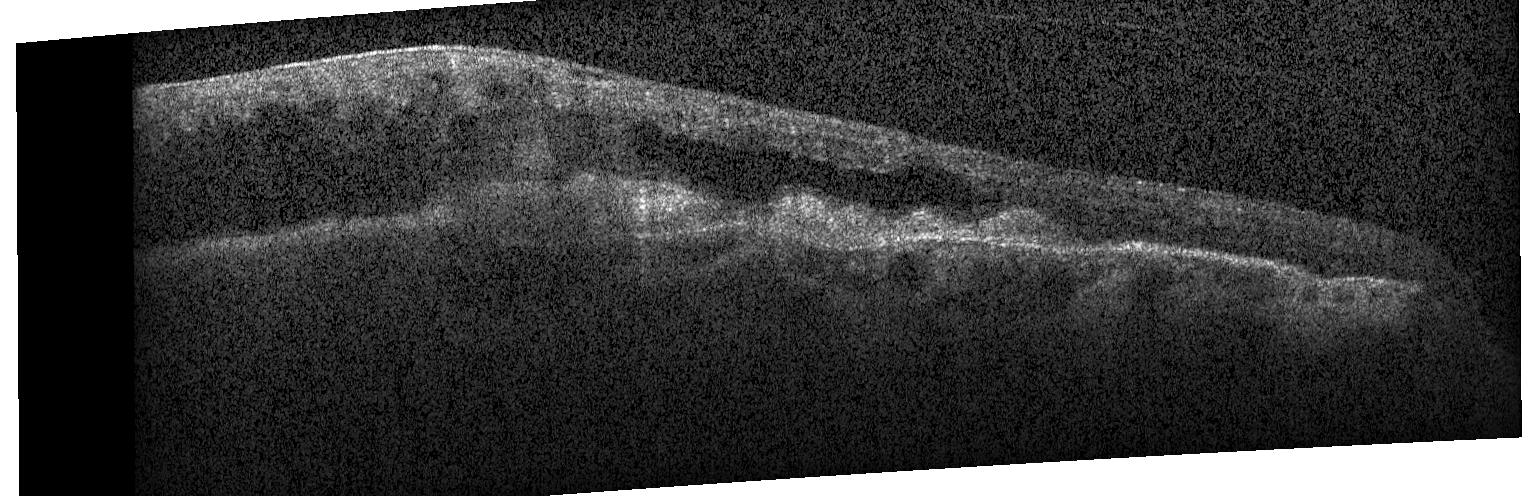 Macular OCT: CNV.